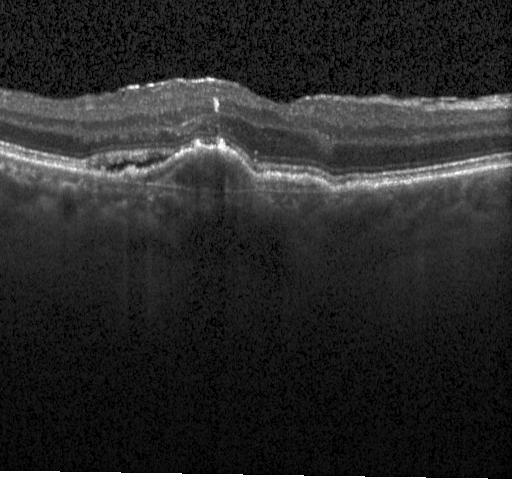
Spectral-domain optical coherence tomography, instrument: Heidelberg Spectralis, optical coherence tomography scan, fovea-centered.
Impression: a choroidal neovascular membrane.